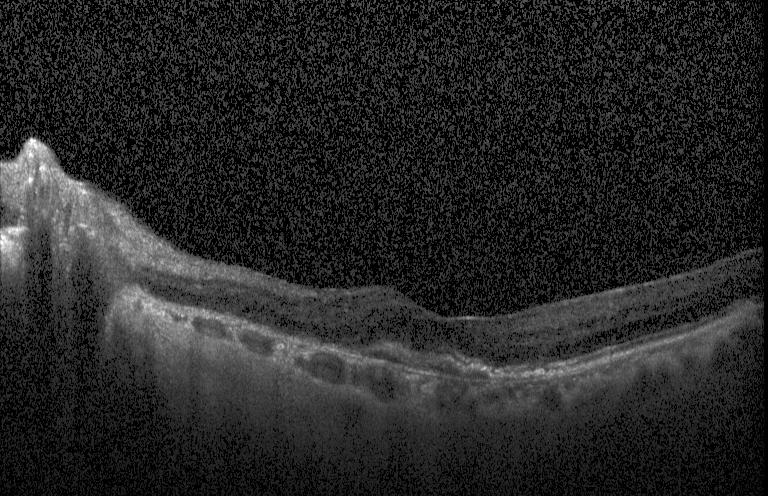
Macular OCT demonstrating a choroidal neovascular membrane.